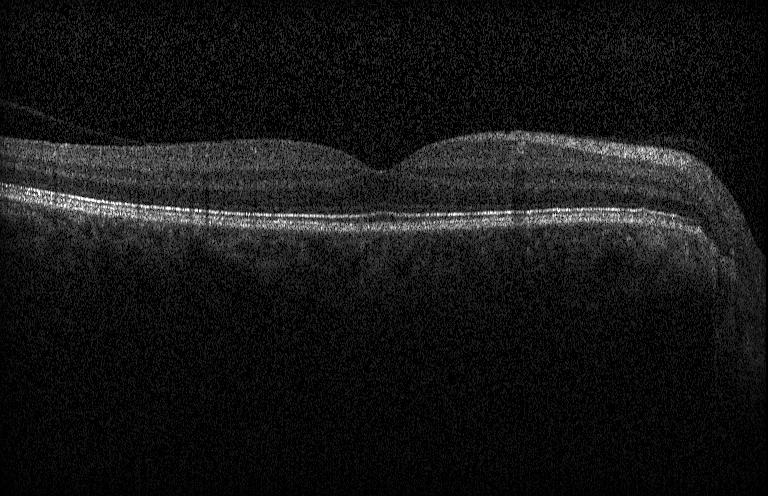

Optical coherence tomography B-scan, acquired on a Heidelberg Spectralis
Macular OCT: no choroidal neovascularization, no diabetic macular edema, and no drusen.